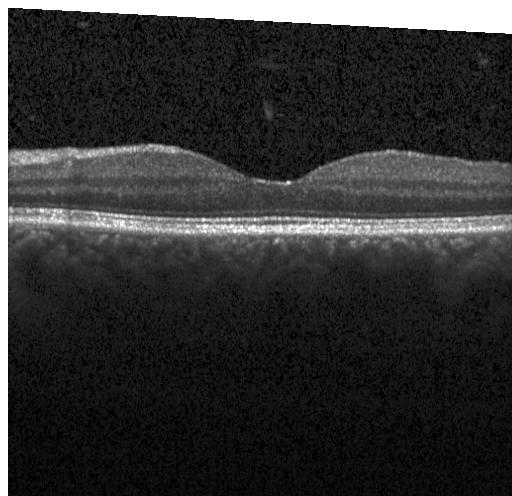 Impression: no CNV, no DME, and no drusen.